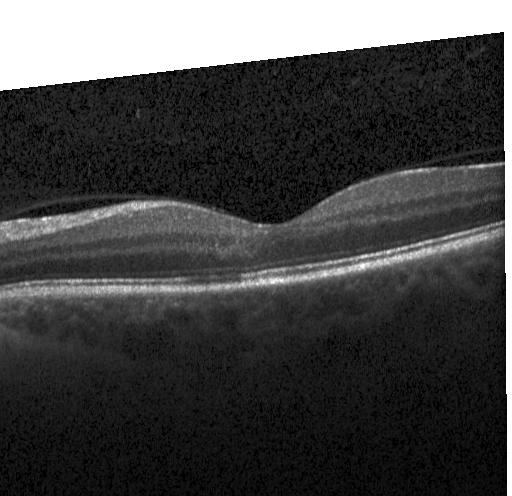 Dx: no evidence of choroidal neovascularization, diabetic macular edema, or drusen.